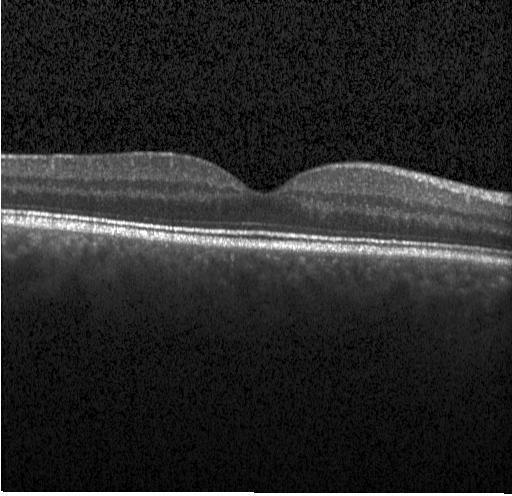 Horizontal scan through the fovea. Retinal OCT cross-section — OCT finding: no CNV, no DME, and no drusen.